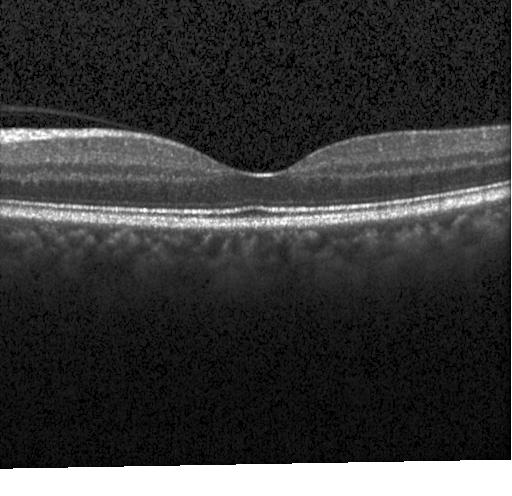
Centered on the fovea. OCT line scan — This B-scan demonstrates neither choroidal neovascularization, diabetic macular edema, nor drusen.